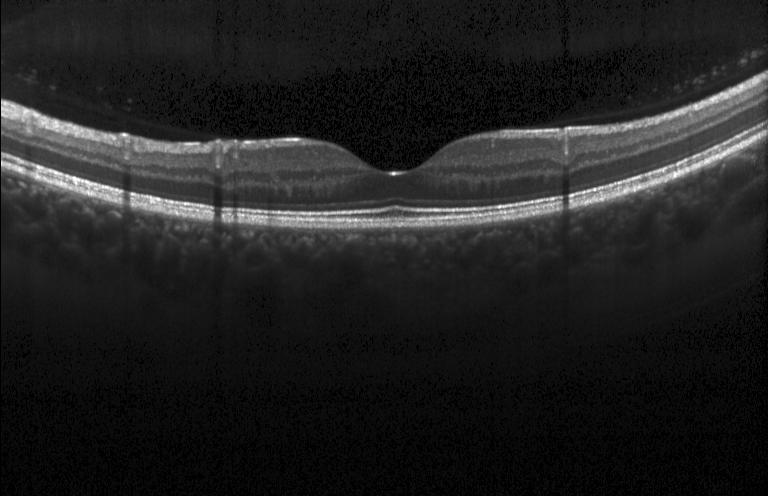
Retinal OCT cross-section — Finding: no CNV, no DME, and no drusen.